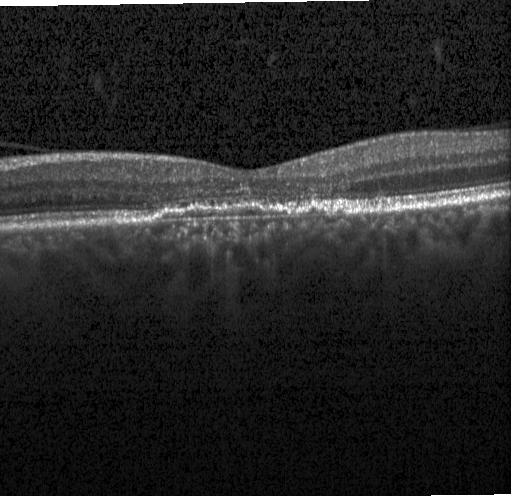 Fovea-centered. OCT B-scan. Impression: choroidal neovascularization (CNV).